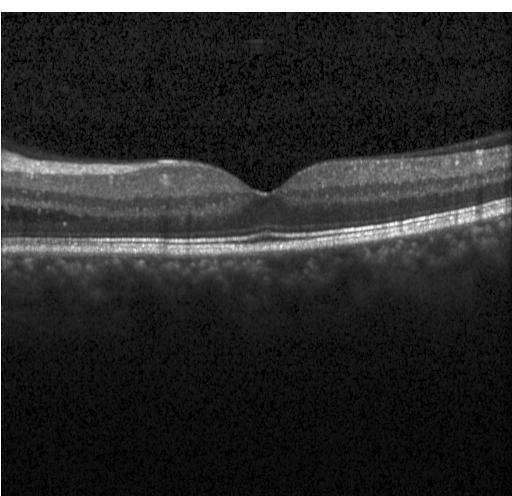
Macular OCT: no choroidal neovascularization, no diabetic macular edema, and no drusen.